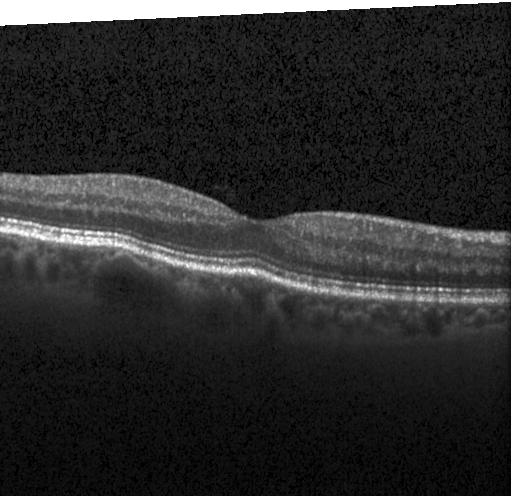

Retinal OCT B-scan.
Neither CNV, DME, nor drusen.